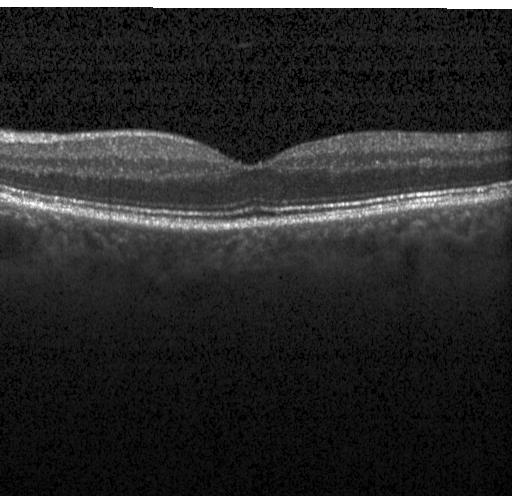 Retinal OCT cross-section showing no CNV, no DME, and no drusen.